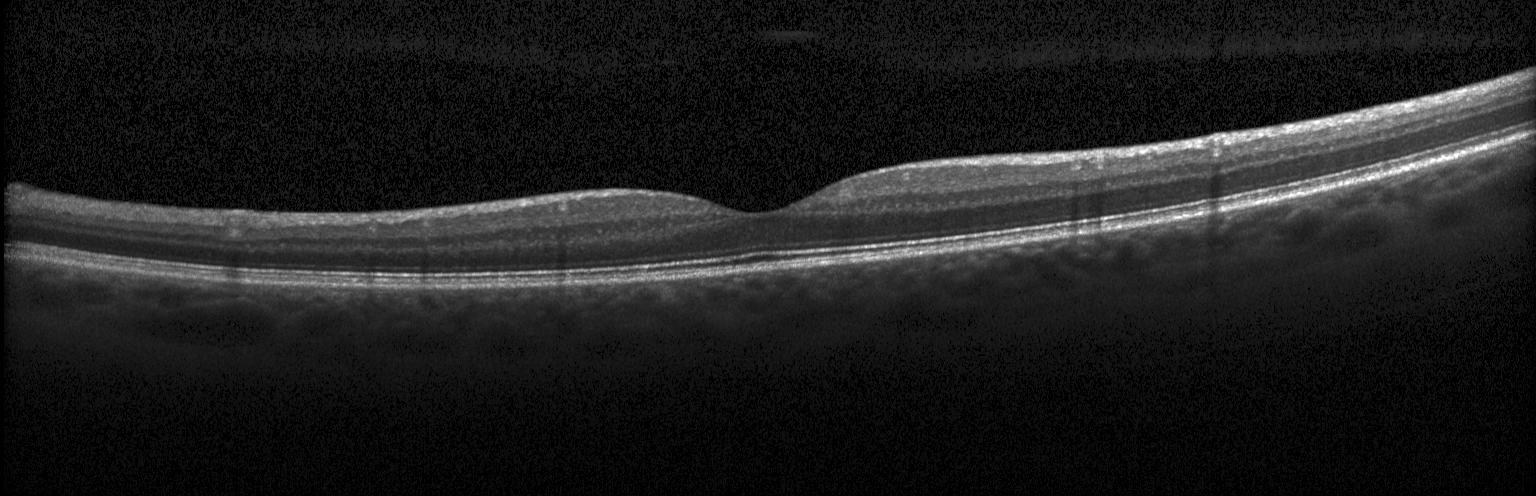

Neither choroidal neovascularization, diabetic macular edema, nor drusen.